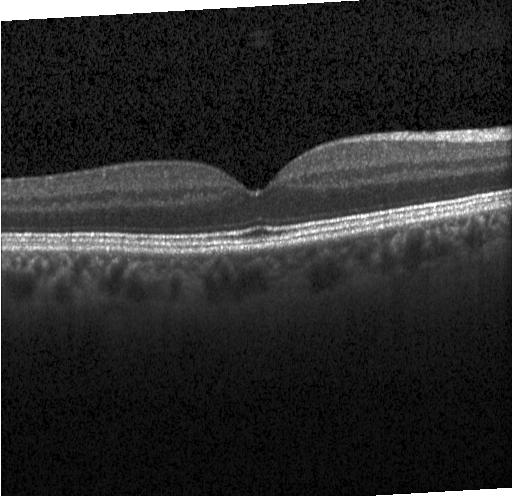

Fovea-centered; optical coherence tomography B-scan; instrument: Heidelberg Spectralis. Diagnosis: no CNV, no DME, and no drusen.